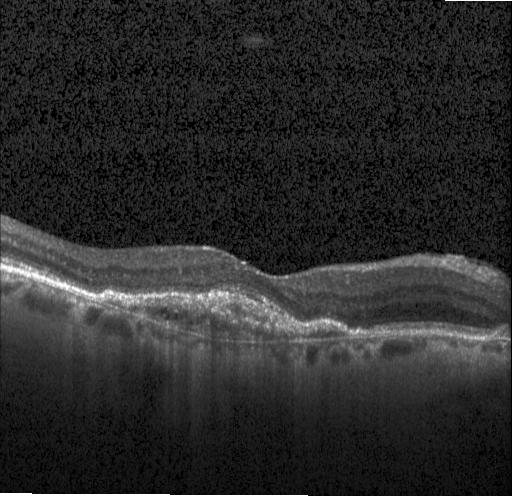
Choroidal neovascularization (CNV).